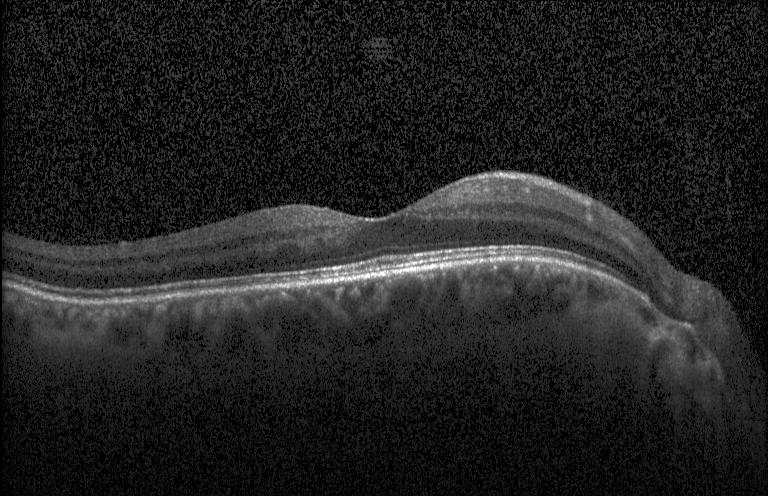 Finding: no choroidal neovascularization, diabetic macular edema, or drusen.